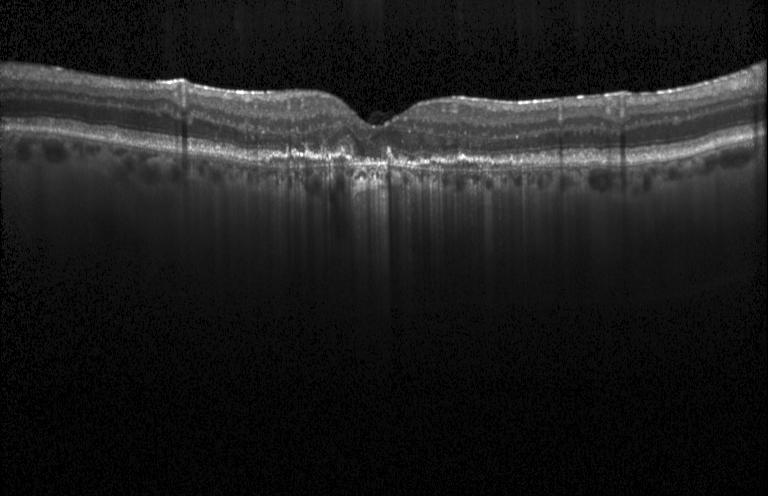

Through the macula · retinal OCT cross-section
Macular OCT: a choroidal neovascular membrane.